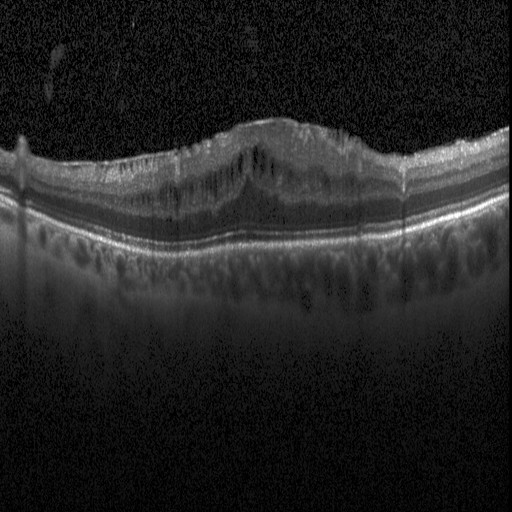

Heidelberg Spectralis; optical coherence tomography scan; fovea-centered — DME.